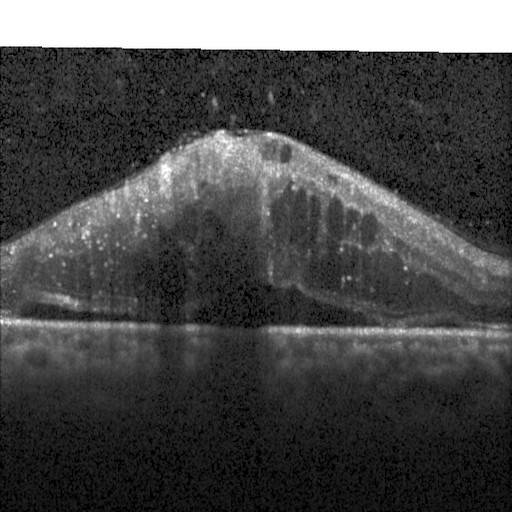

OCT line scan; Heidelberg Spectralis; macular scan
Diagnosis: diabetic macular edema (DME).